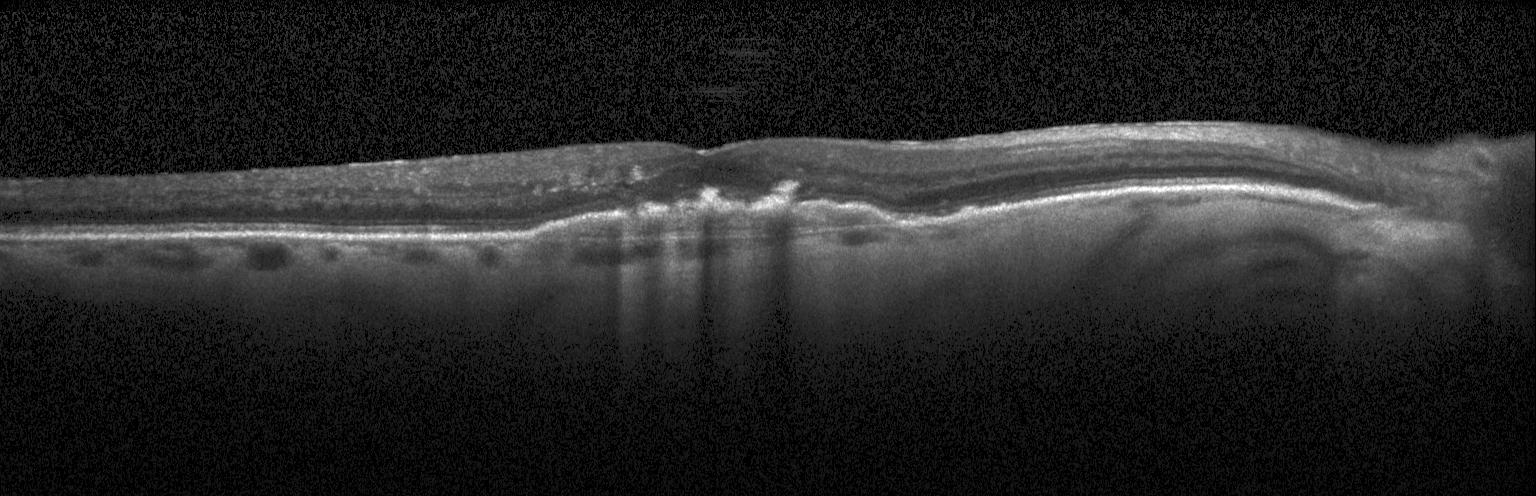 OCT B-scan showing choroidal neovascularization (CNV).